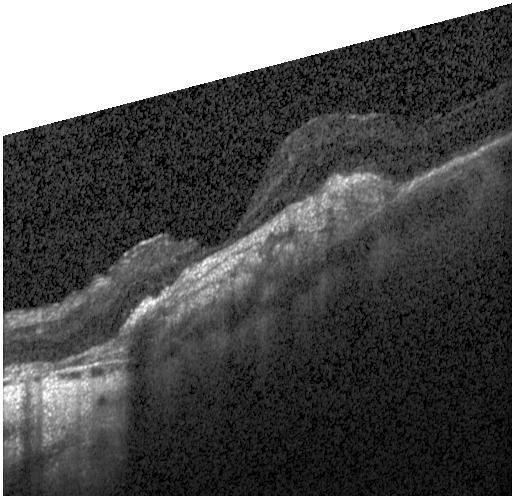

Horizontal scan through the fovea · optical coherence tomography scan · spectral-domain OCT · instrument: Heidelberg Spectralis. Diagnosis: choroidal neovascularization (CNV).